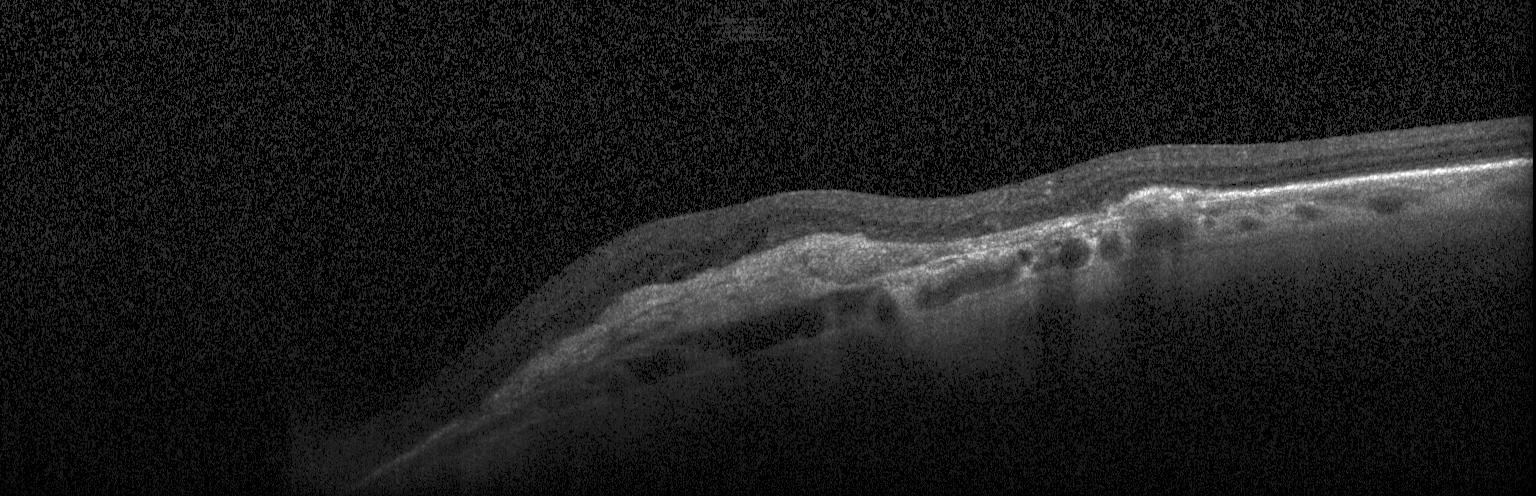

Finding: a choroidal neovascular membrane.